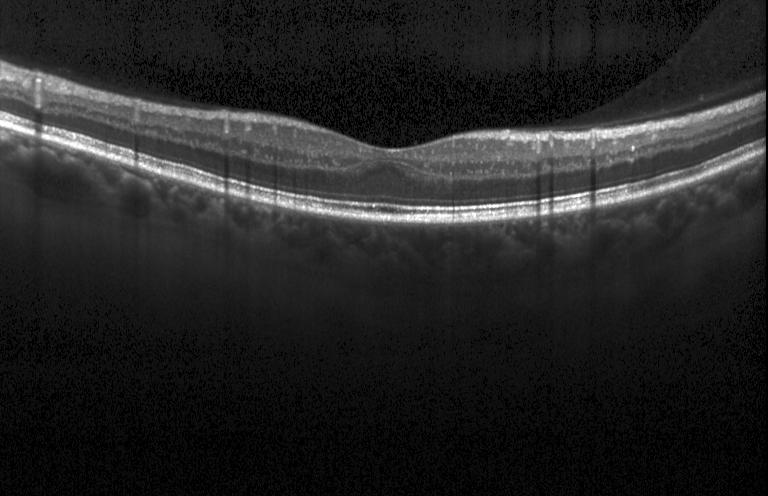 OCT B-scan showing neither CNV, DME, nor drusen.